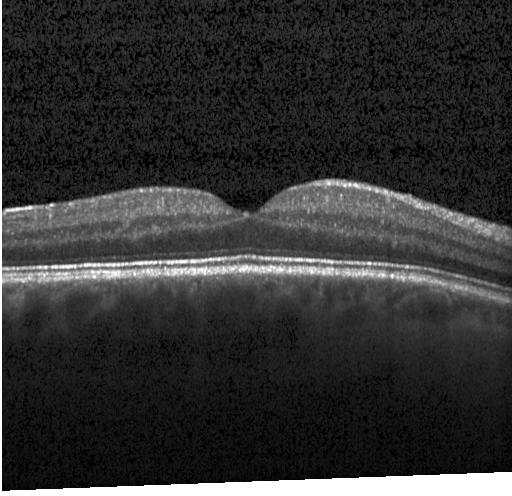 SD-OCT, retinal OCT B-scan, horizontal scan through the fovea, Heidelberg Spectralis OCT system. Impression: no CNV, DME, or drusen.